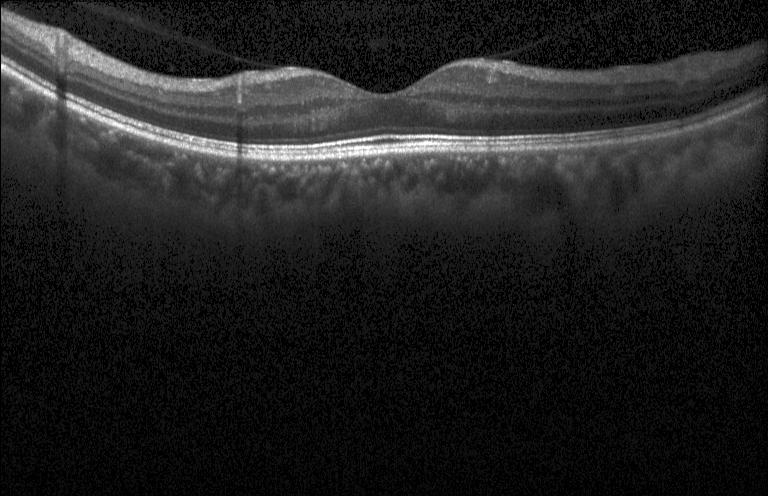 Retinal OCT B-scan — Dx: no CNV, no DME, and no drusen.